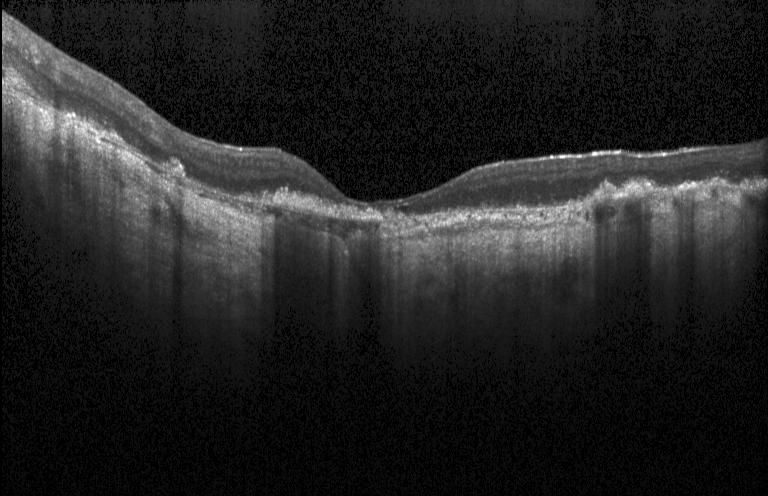 Spectral-domain optical coherence tomography · Heidelberg Spectralis OCT system · OCT line scan · centered on the fovea. Macular OCT: CNV.